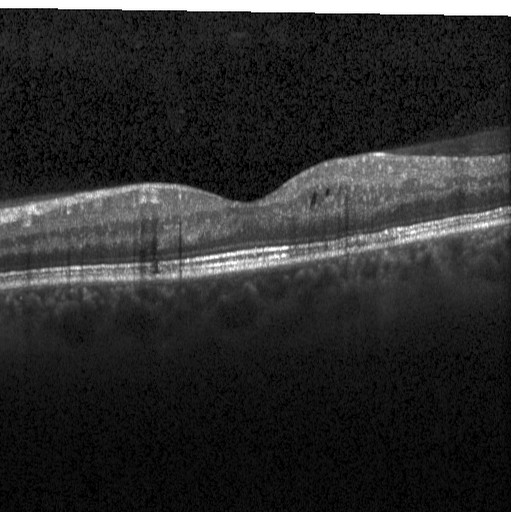 OCT scan showing diabetic macular edema.